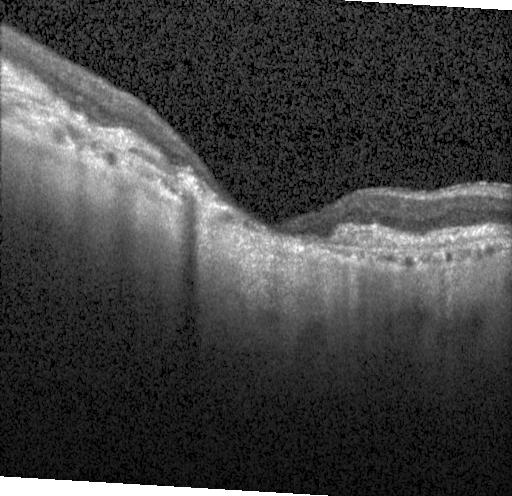
Optical coherence tomography B-scan. Finding: CNV.